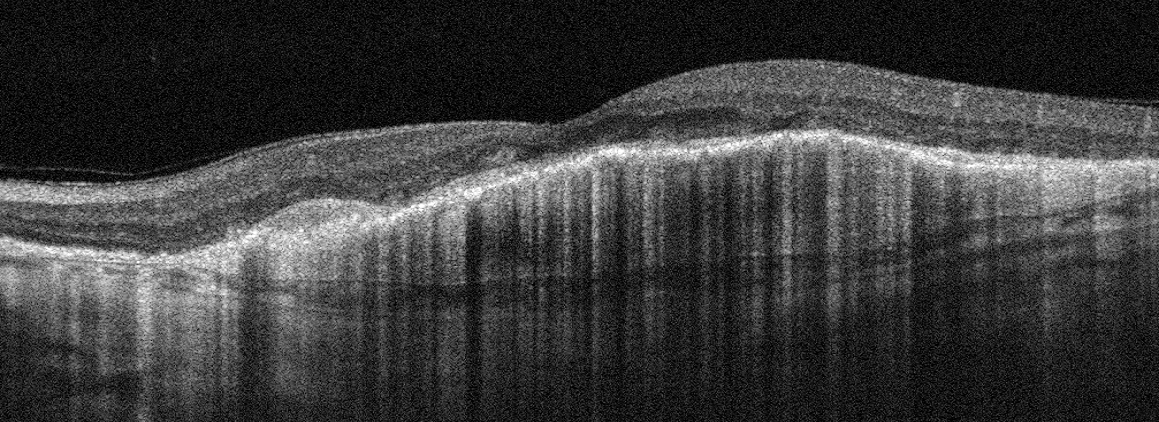
OS; optical coherence tomography scan. Age-related macular degeneration (AMD).